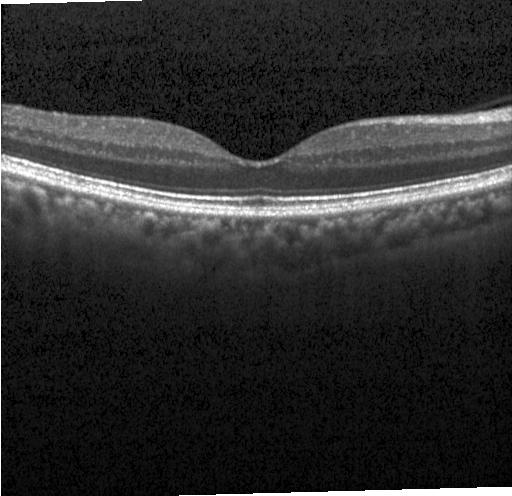

Heidelberg Spectralis OCT system. Spectral-domain optical coherence tomography. OCT line scan. Horizontal scan through the fovea. Impression: no evidence of choroidal neovascularization, diabetic macular edema, or drusen.